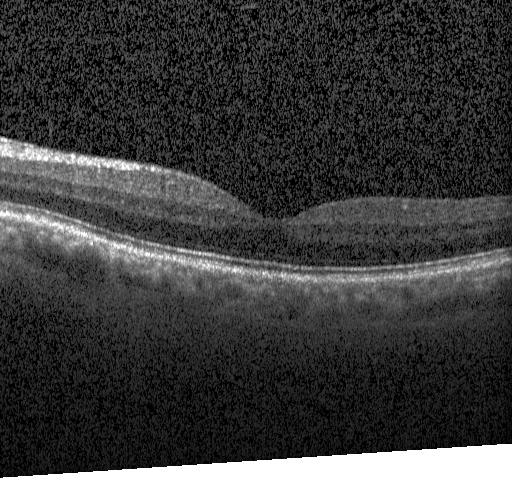

Retinal OCT cross-section; spectral-domain OCT; acquired on a Heidelberg Spectralis.
Dx: no choroidal neovascularization, diabetic macular edema, or drusen.